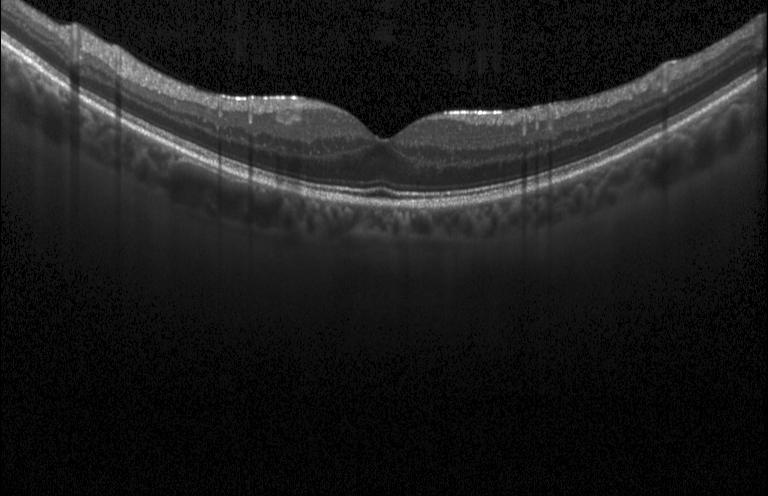
Diagnosis: no evidence of choroidal neovascularization, diabetic macular edema, or drusen.